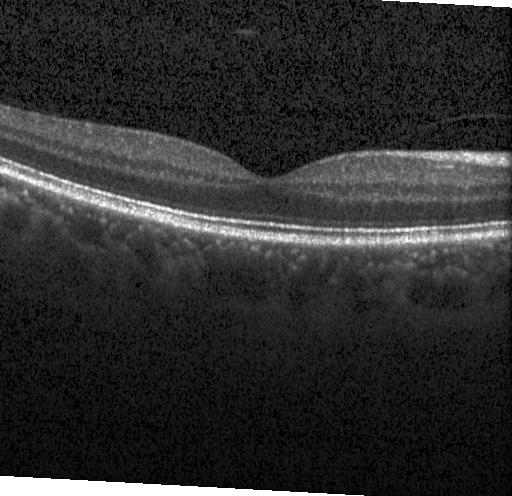
OCT B-scan; fovea-centered — Dx: neither choroidal neovascularization, diabetic macular edema, nor drusen.